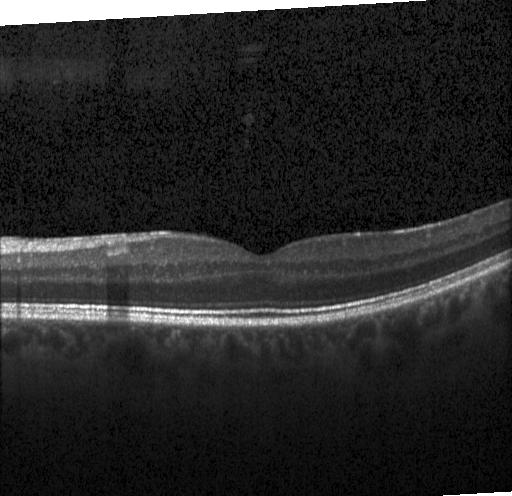
No evidence of choroidal neovascularization, diabetic macular edema, or drusen.